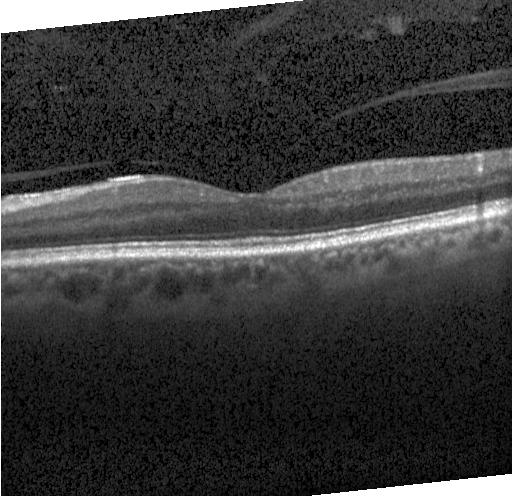
Optical coherence tomography B-scan; centered on the fovea. Diagnosis: no CNV, DME, or drusen.